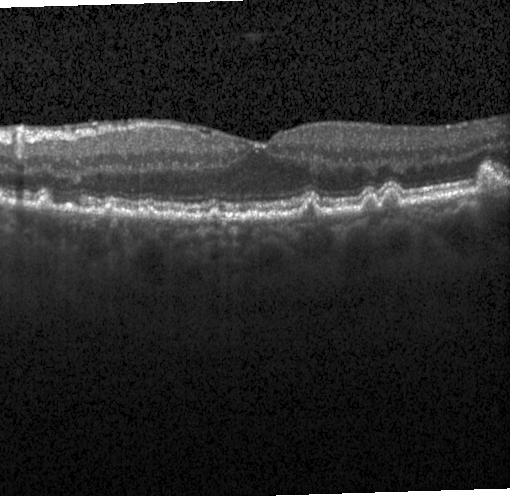
OCT B-scan. Dx: multiple drusen.